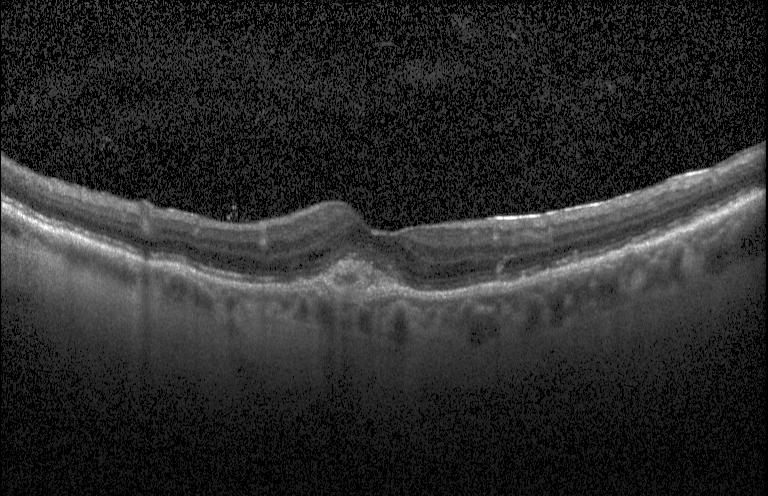

Finding: choroidal neovascularization (CNV).